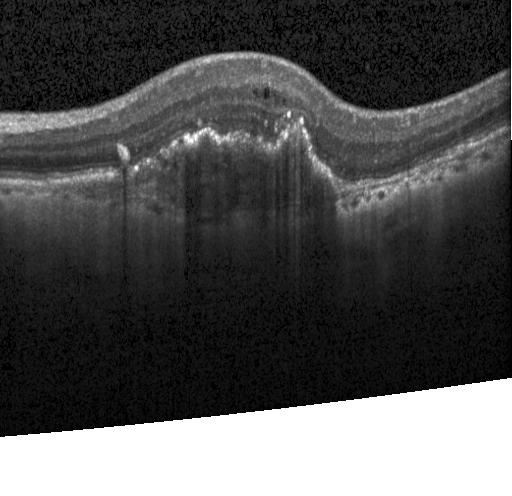
Spectral-domain OCT; acquired on a Heidelberg Spectralis; macular scan; OCT B-scan. OCT finding: CNV.